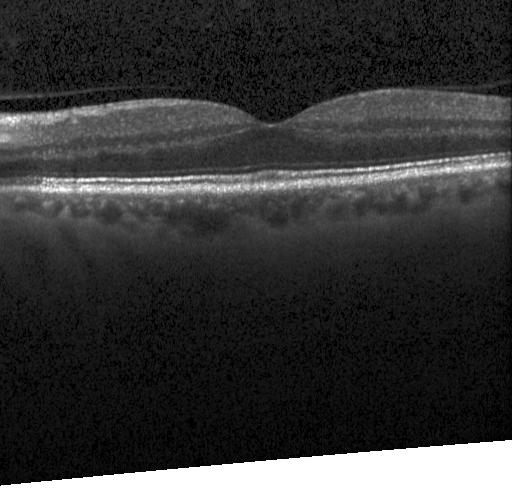

OCT scan showing no choroidal neovascularization, diabetic macular edema, or drusen.